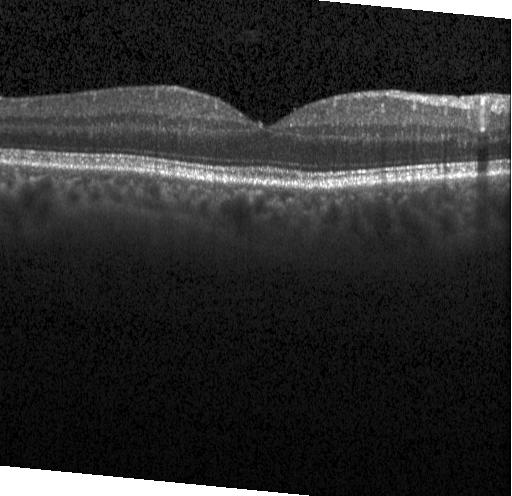

Finding: no choroidal neovascularization, no diabetic macular edema, and no drusen.